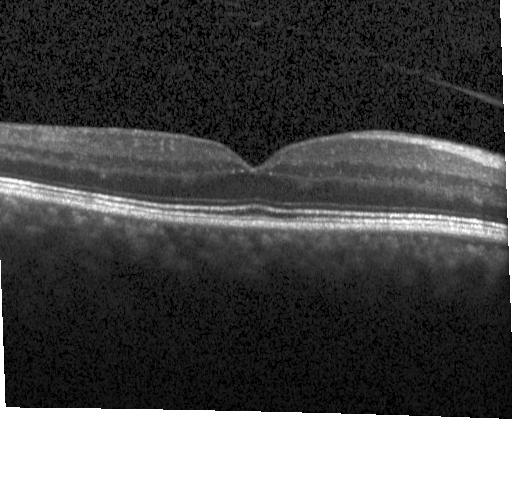 OCT B-scan — This B-scan demonstrates no evidence of choroidal neovascularization, diabetic macular edema, or drusen.